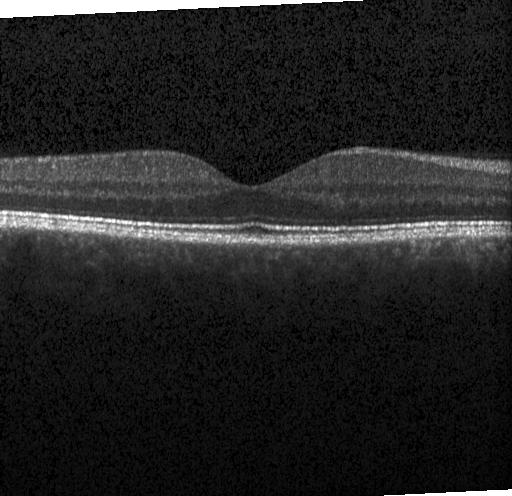

Heidelberg Spectralis, OCT B-scan
Impression: no evidence of choroidal neovascularization, diabetic macular edema, or drusen.